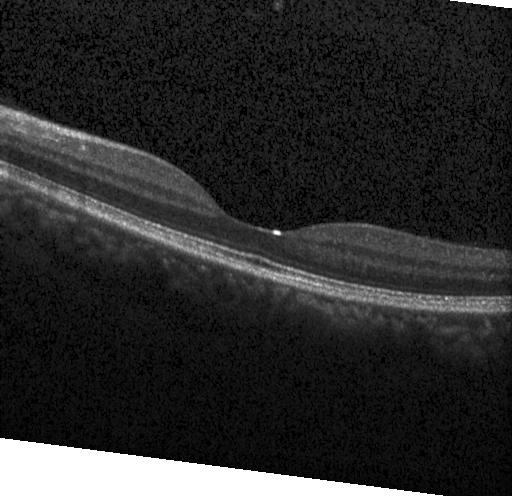 Horizontal scan through the fovea; instrument: Heidelberg Spectralis; spectral-domain OCT; retinal OCT cross-section — Diagnosis: neither choroidal neovascularization, diabetic macular edema, nor drusen.